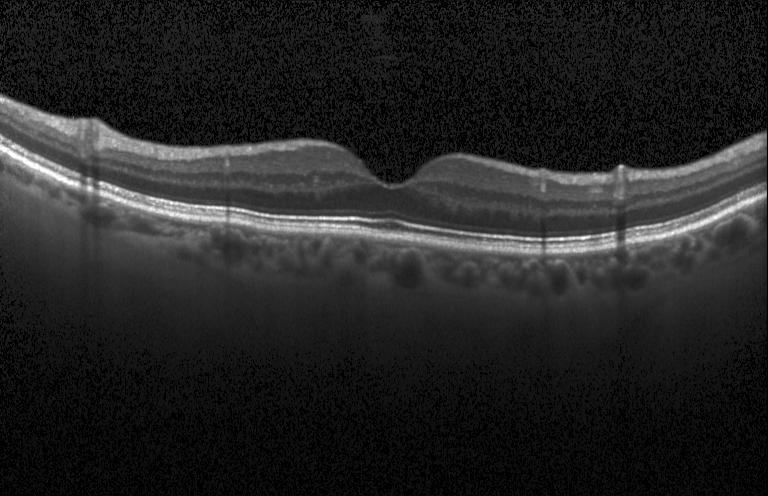

Optical coherence tomography scan.
Assessment: no CNV, DME, or drusen.